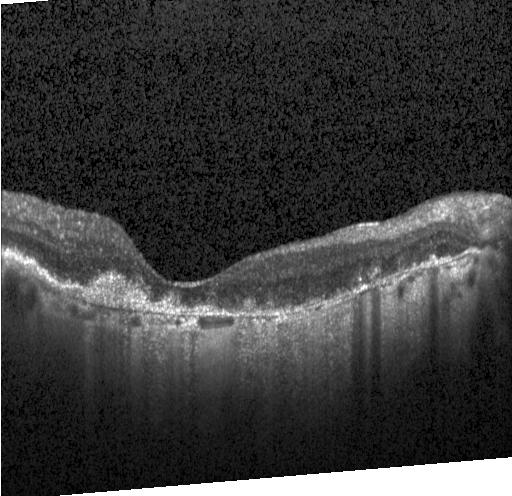 A choroidal neovascular membrane.